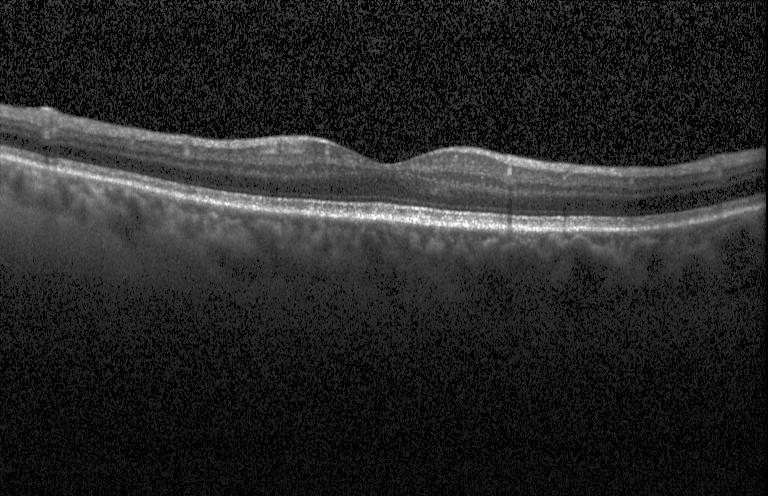
Heidelberg Spectralis · OCT line scan — Macular OCT: no choroidal neovascularization, no diabetic macular edema, and no drusen.